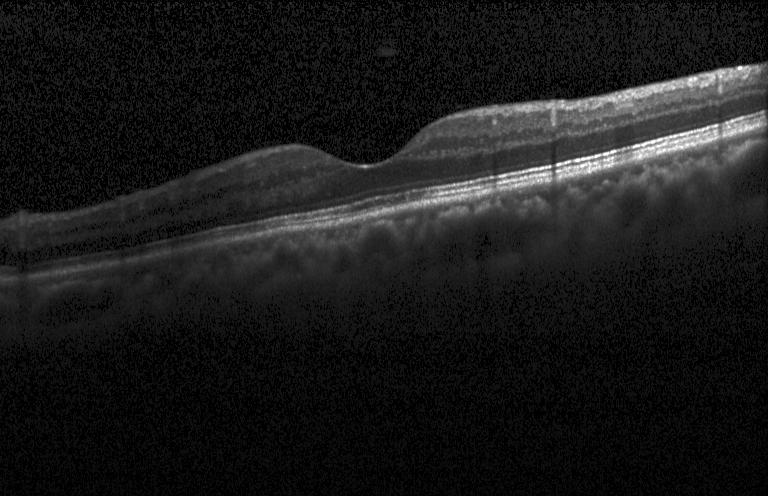

Optical coherence tomography B-scan — Diagnosis: no choroidal neovascularization, no diabetic macular edema, and no drusen.